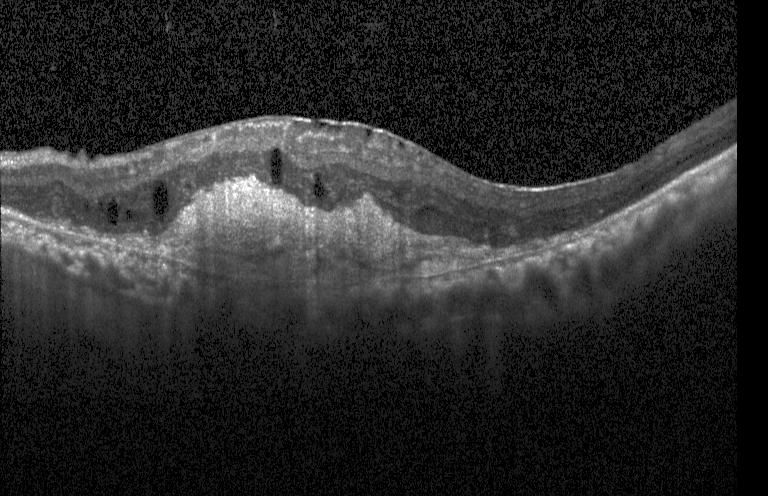 SD-OCT. Retinal OCT B-scan. Macular scan. Heidelberg Spectralis — Dx: a choroidal neovascular membrane.